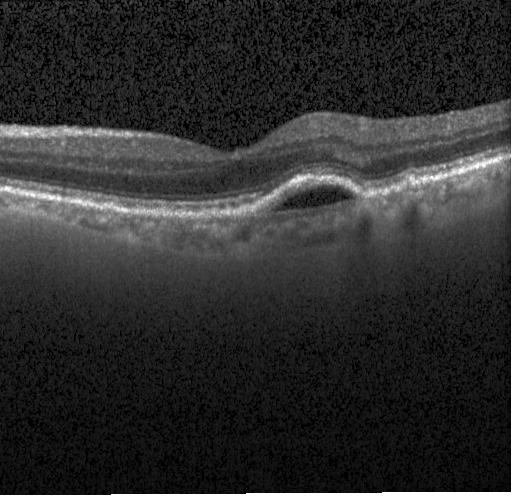
Diagnosis: a choroidal neovascular membrane.